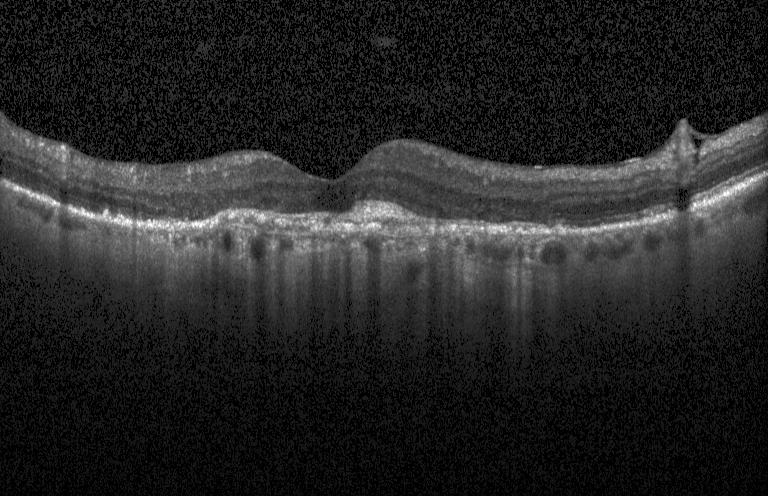

OCT scan showing a choroidal neovascular membrane.